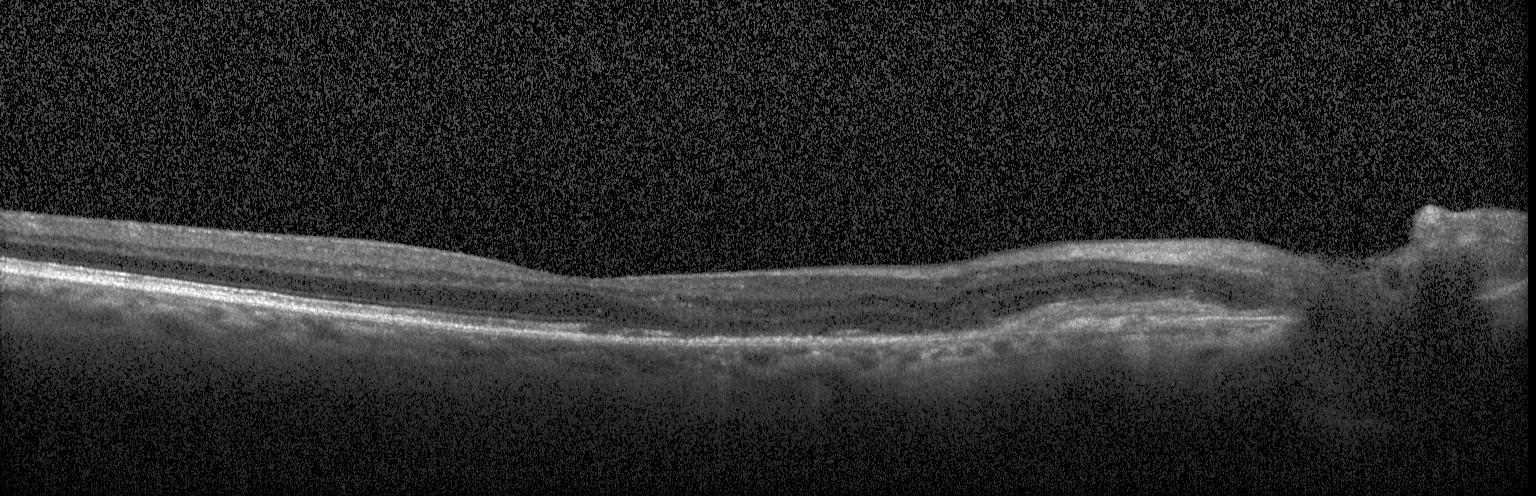

Retinal OCT cross-section showing choroidal neovascularization.